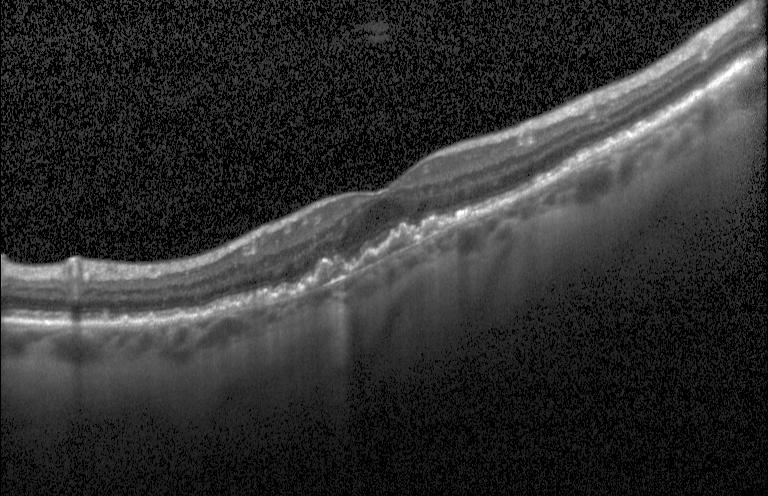 OCT B-scan. Finding: a choroidal neovascular membrane.